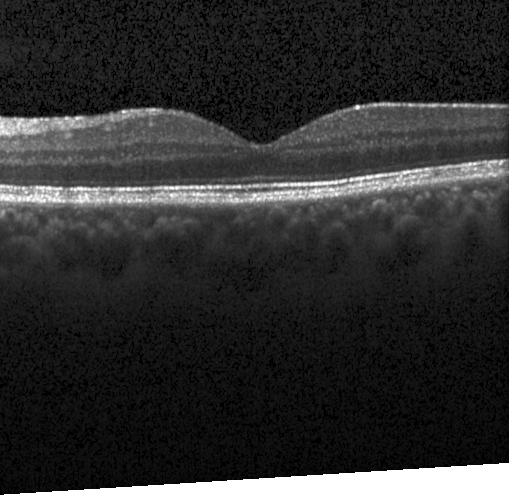 Retinal OCT cross-section, macular scan
Impression: neither choroidal neovascularization, diabetic macular edema, nor drusen.